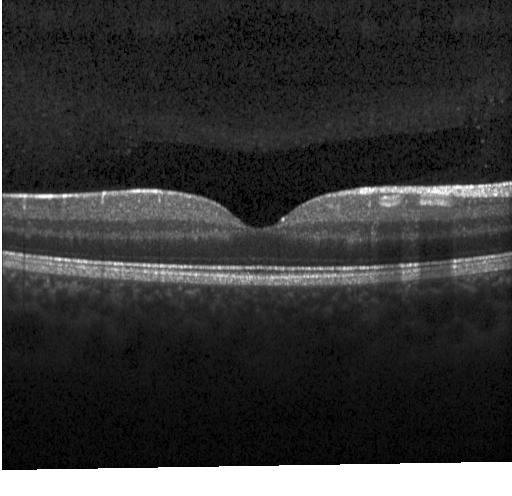
OCT line scan — Finding: neither choroidal neovascularization, diabetic macular edema, nor drusen.